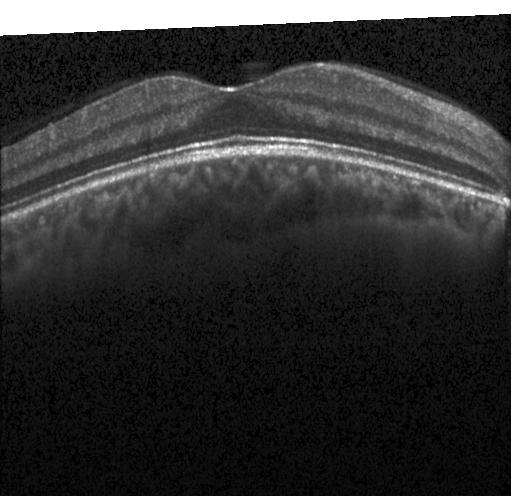

Finding: neither choroidal neovascularization, diabetic macular edema, nor drusen.